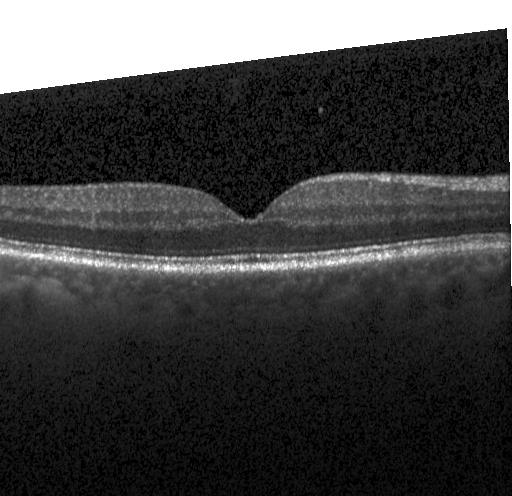

Finding: no choroidal neovascularization, diabetic macular edema, or drusen.